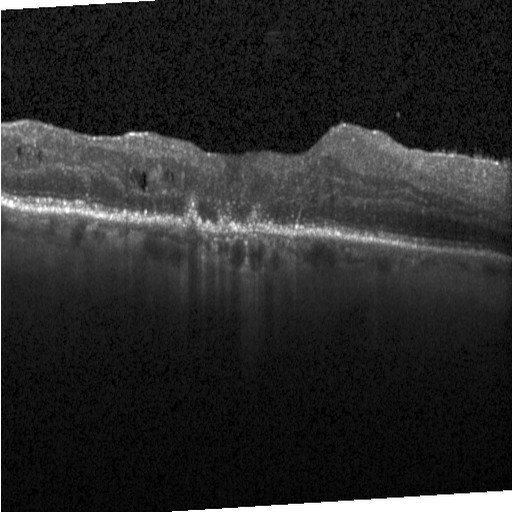 Instrument: Heidelberg Spectralis. Retinal OCT B-scan
This B-scan demonstrates DME.